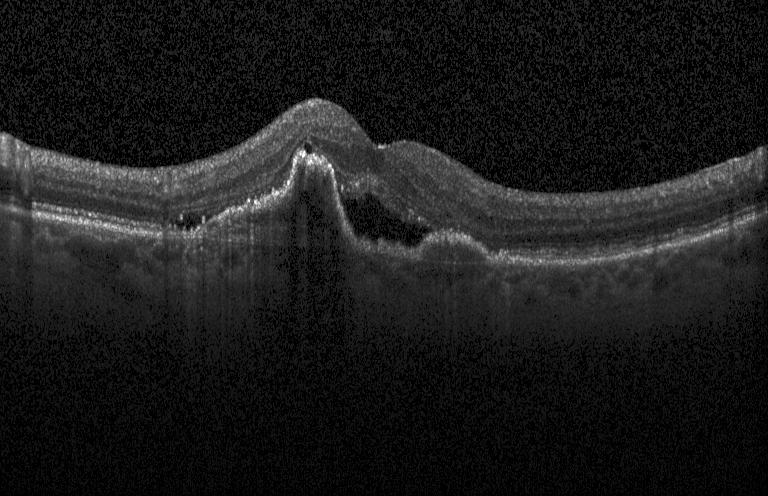

Retinal OCT cross-section. Spectral-domain OCT. Assessment: a choroidal neovascular membrane.